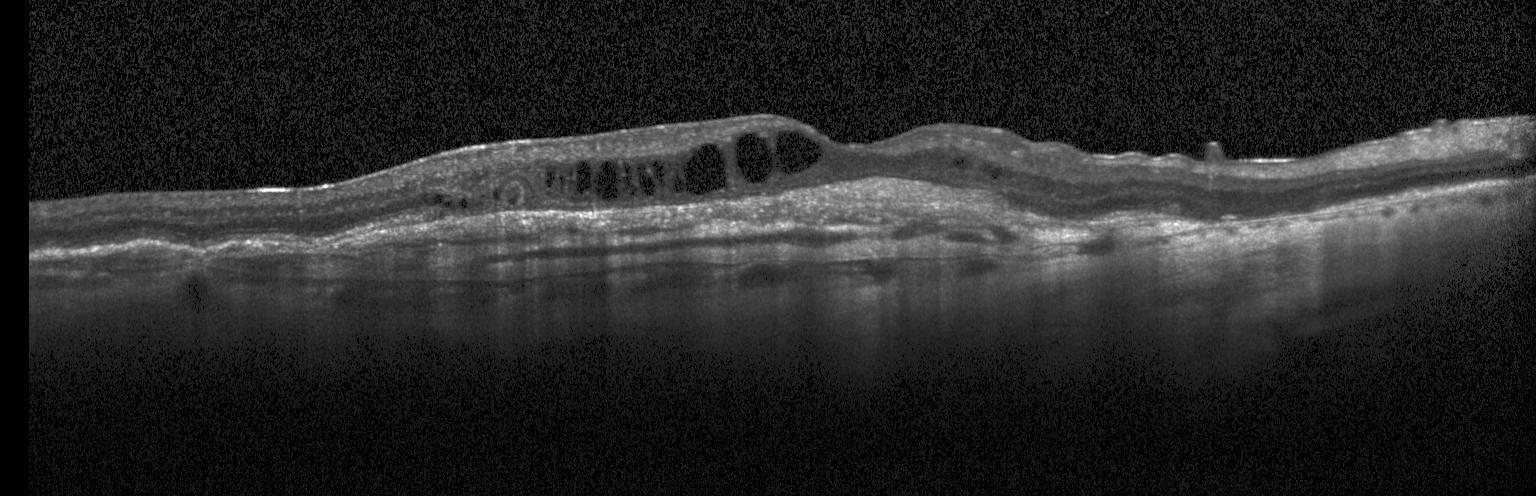
Macular OCT: a choroidal neovascular membrane.